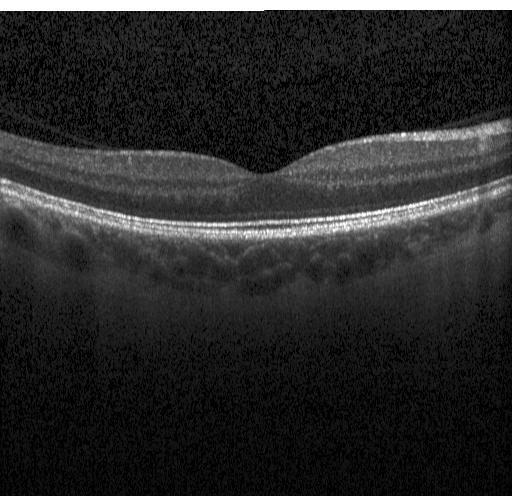

Finding: no evidence of choroidal neovascularization, diabetic macular edema, or drusen.